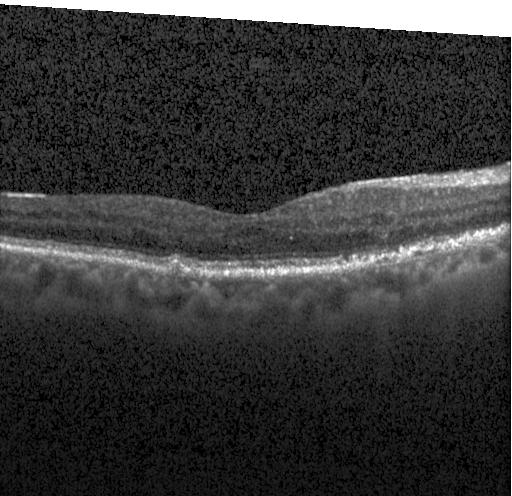
Horizontal scan through the fovea, Heidelberg Spectralis, optical coherence tomography B-scan, SD-OCT — Multiple drusen.